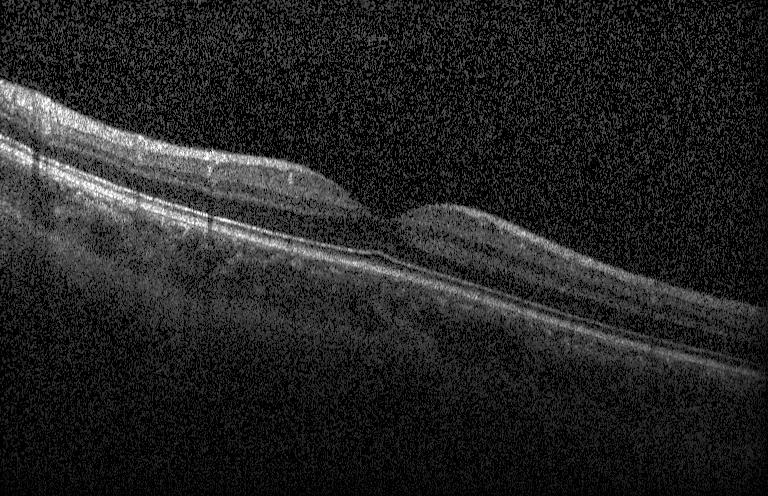

Optical coherence tomography scan · instrument: Heidelberg Spectralis — Macular OCT: no choroidal neovascularization, diabetic macular edema, or drusen.